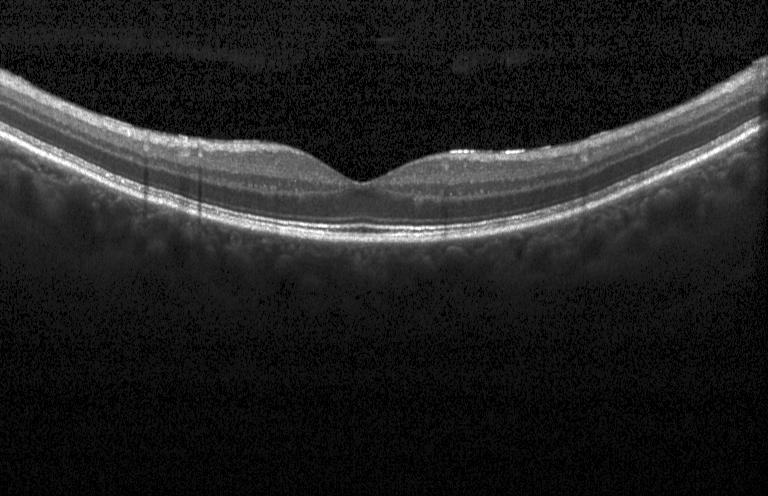

OCT scan showing neither CNV, DME, nor drusen.